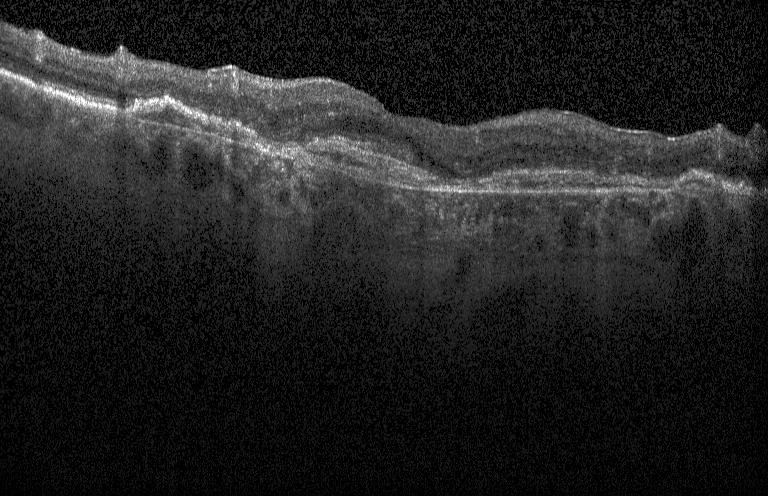

Macular OCT: a choroidal neovascular membrane.